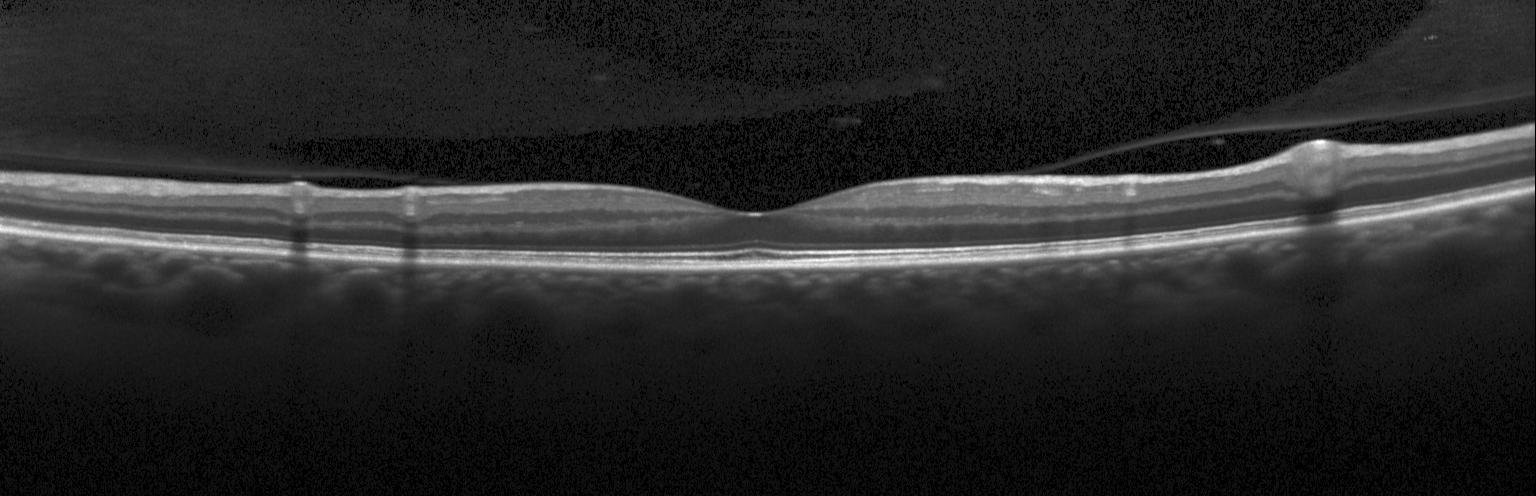
OCT line scan, instrument: Heidelberg Spectralis — Finding: neither choroidal neovascularization, diabetic macular edema, nor drusen.